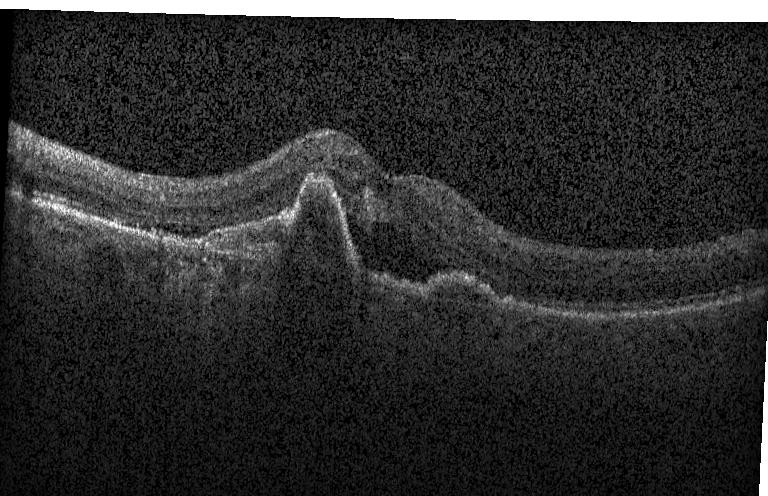

OCT scan showing a choroidal neovascular membrane.